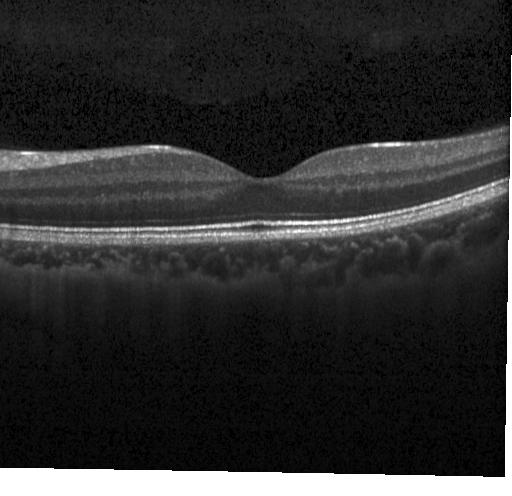 OCT scan showing no evidence of CNV, DME, or drusen.